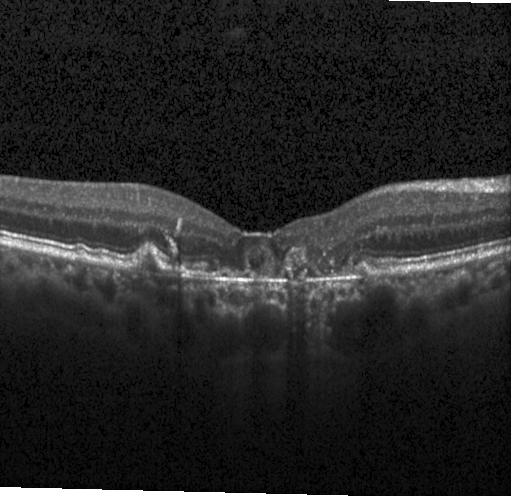 Optical coherence tomography B-scan
Impression: a choroidal neovascular membrane.